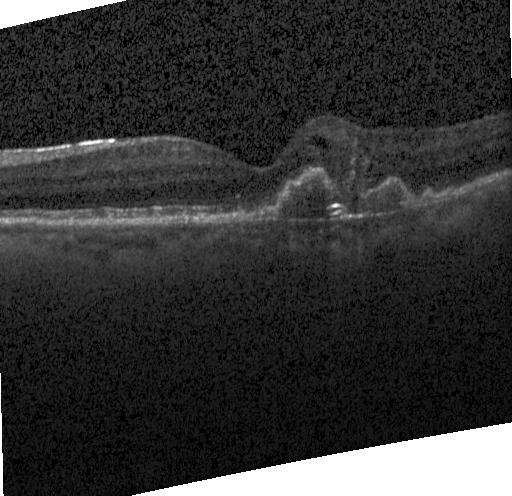

OCT finding: CNV.